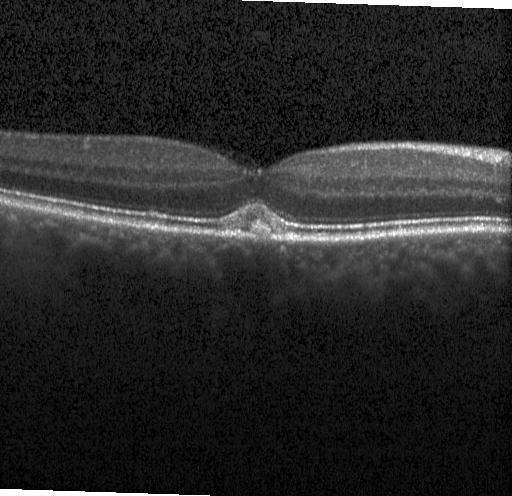
Impression: CNV.